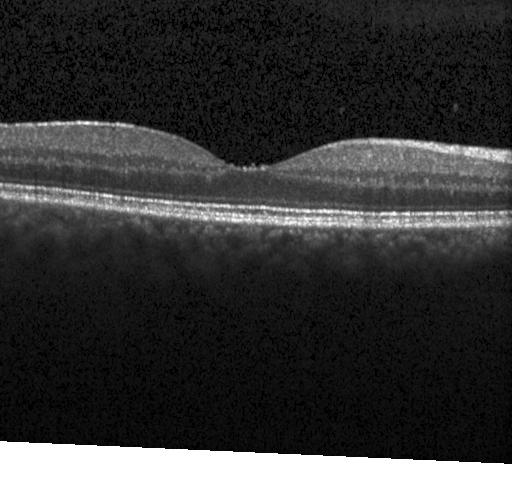

Macular OCT demonstrating no CNV, DME, or drusen.